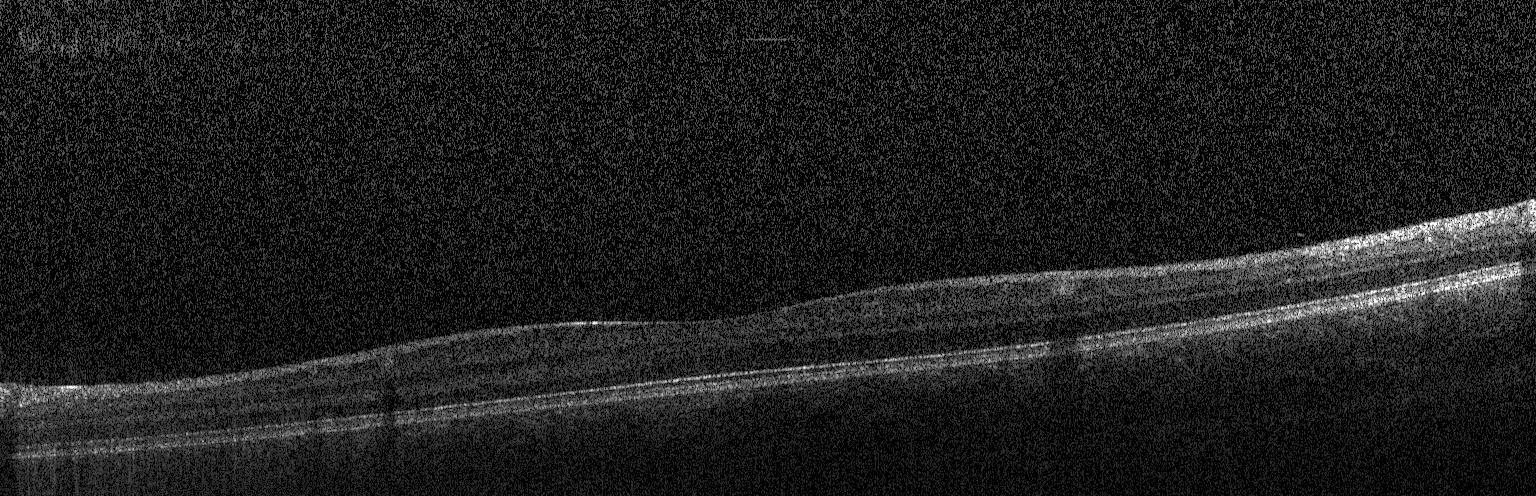

SD-OCT. Optical coherence tomography scan. Horizontal scan through the fovea. Instrument: Heidelberg Spectralis
Impression: no evidence of choroidal neovascularization, diabetic macular edema, or drusen.